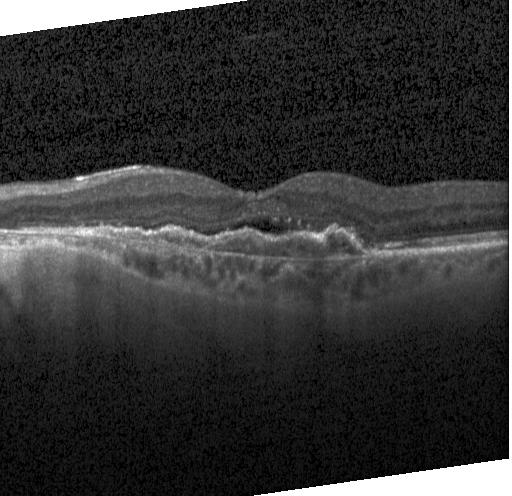

Impression: CNV.